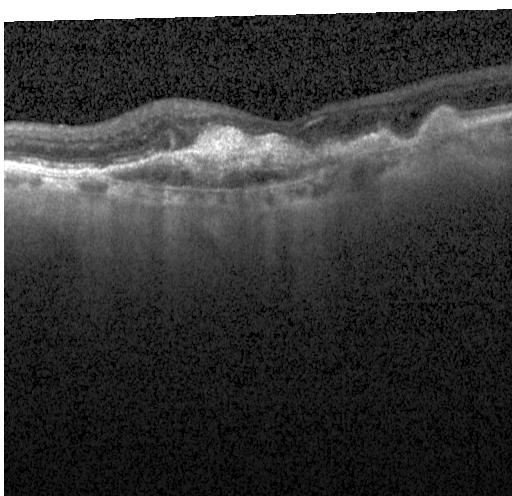
Acquired on a Heidelberg Spectralis · fovea-centered · spectral-domain optical coherence tomography · optical coherence tomography scan
The scan shows choroidal neovascularization (CNV).